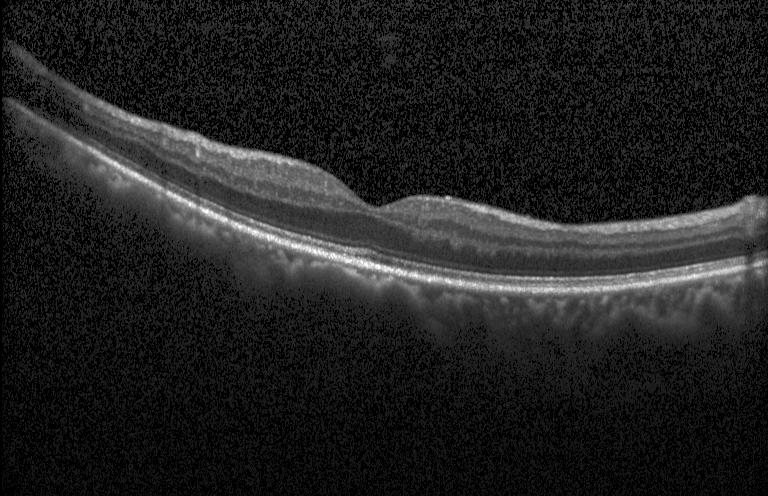 Optical coherence tomography B-scan.
Finding: no choroidal neovascularization, no diabetic macular edema, and no drusen.